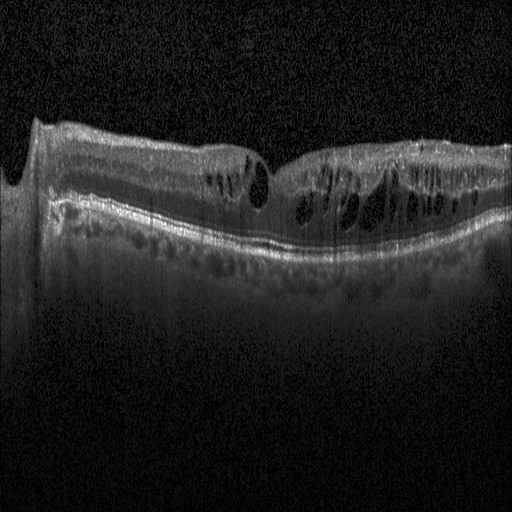
Macular scan, optical coherence tomography B-scan, spectral-domain optical coherence tomography.
Diagnosis: diabetic macular edema (DME).